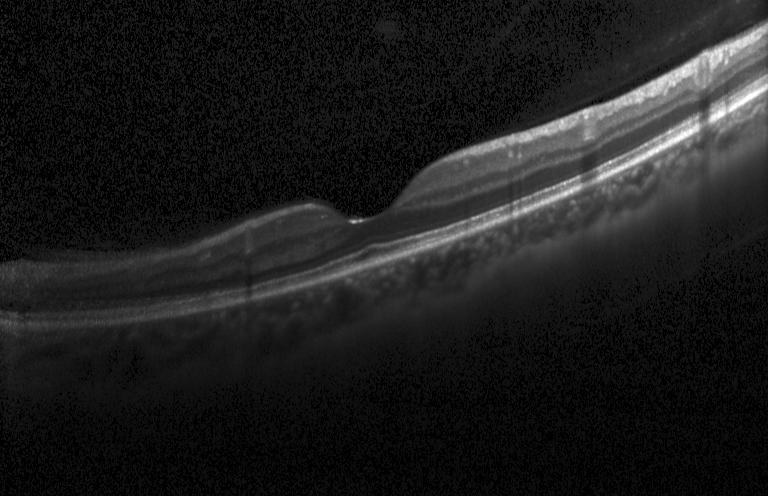

Spectral-domain optical coherence tomography. Instrument: Heidelberg Spectralis. Optical coherence tomography B-scan. Through the macula.
Finding: no choroidal neovascularization, no diabetic macular edema, and no drusen.